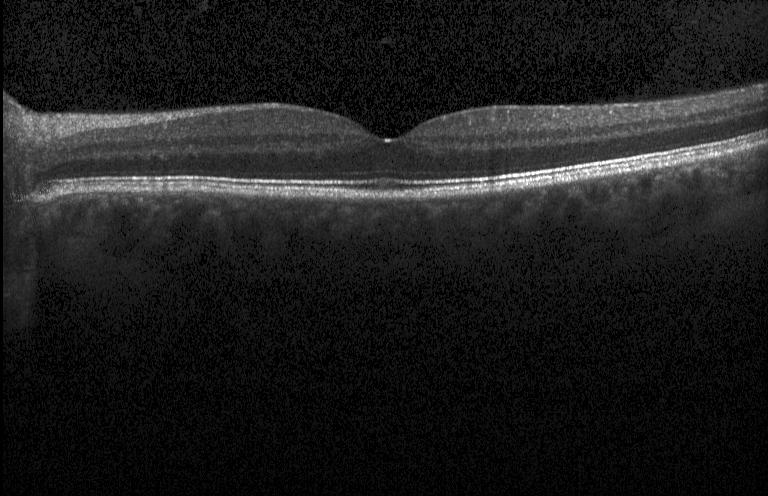

OCT B-scan
The scan shows neither choroidal neovascularization, diabetic macular edema, nor drusen.